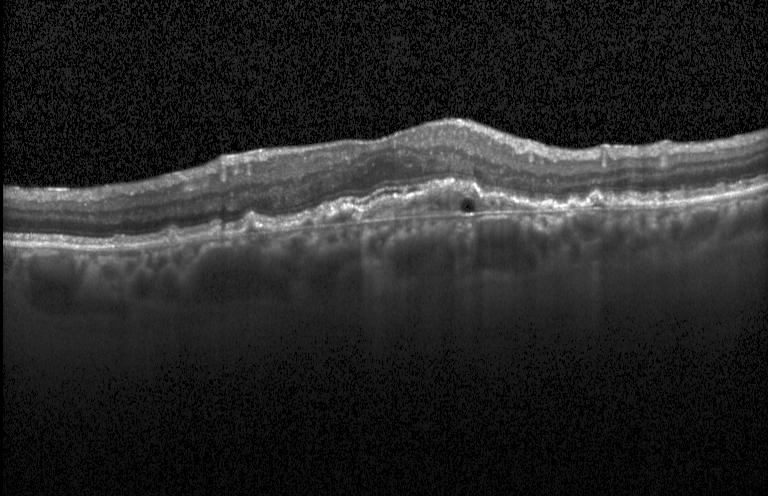

Centered on the fovea, instrument: Heidelberg Spectralis, optical coherence tomography B-scan, spectral-domain OCT.
Dx: choroidal neovascularization.